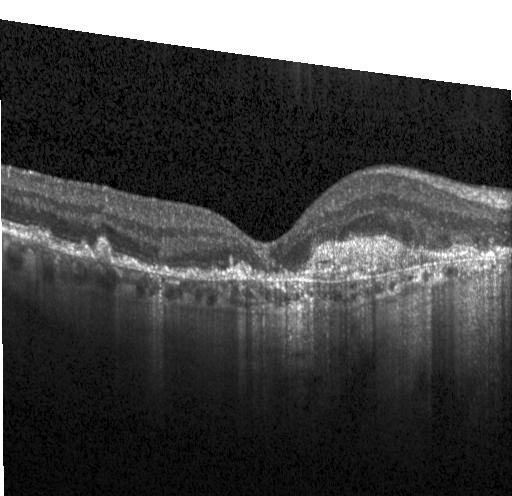

Optical coherence tomography scan
Assessment: CNV.